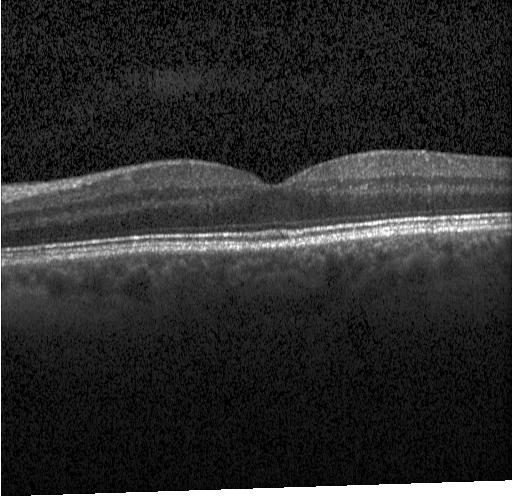

Heidelberg Spectralis OCT system, spectral-domain optical coherence tomography, optical coherence tomography scan, through the macula.
Diagnosis: neither choroidal neovascularization, diabetic macular edema, nor drusen.